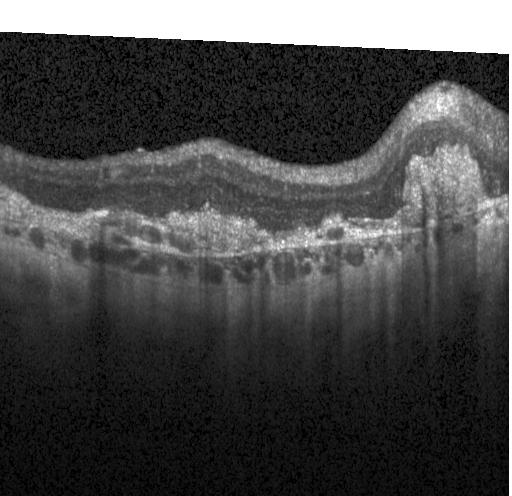 Spectral-domain optical coherence tomography. Retinal OCT cross-section. Diagnosis: a choroidal neovascular membrane.